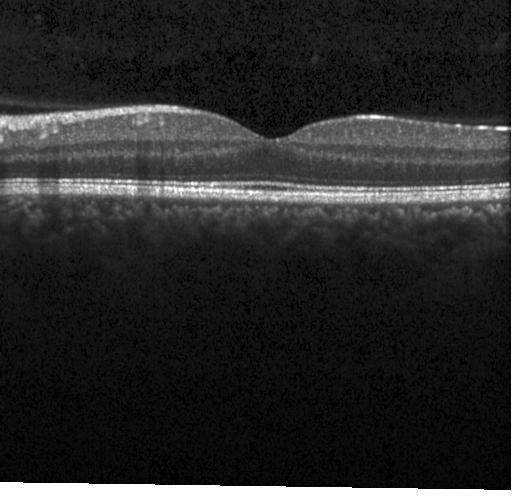 Optical coherence tomography scan — Finding: neither choroidal neovascularization, diabetic macular edema, nor drusen.